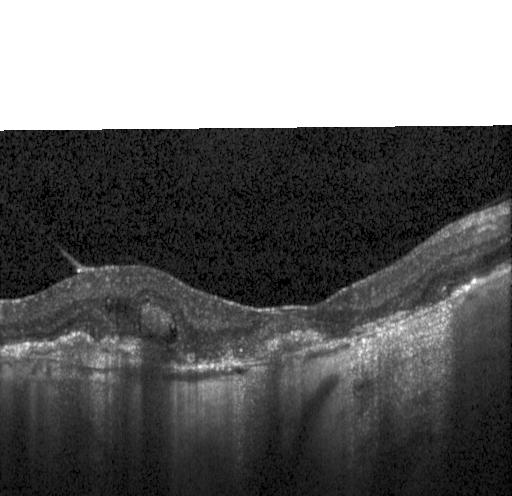
Finding: a choroidal neovascular membrane.